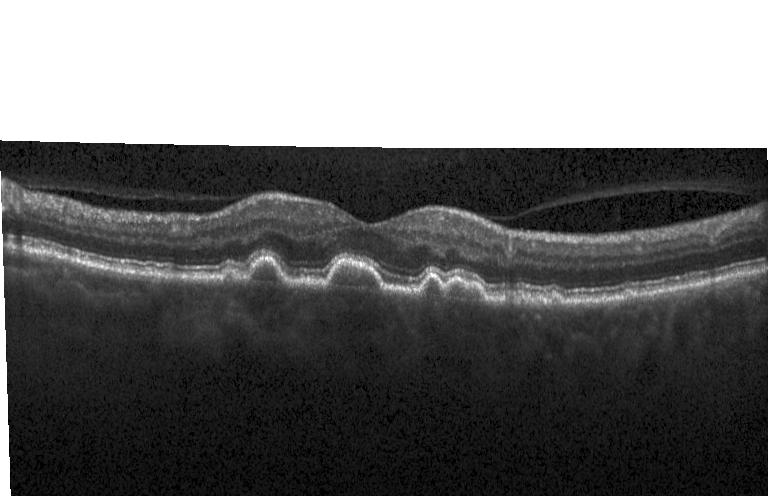

Horizontal scan through the fovea; OCT B-scan
This B-scan demonstrates multiple drusen.